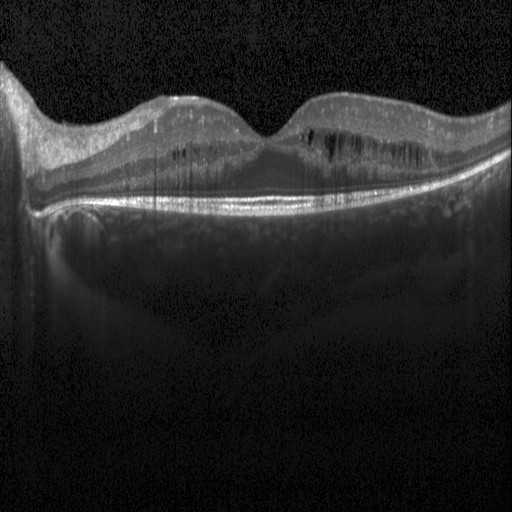
DME.